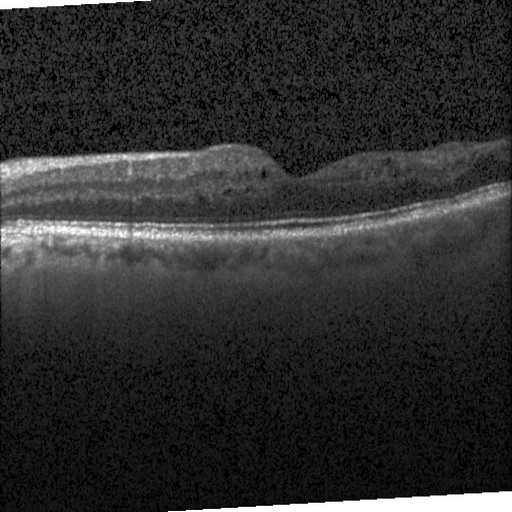
Impression: DME.